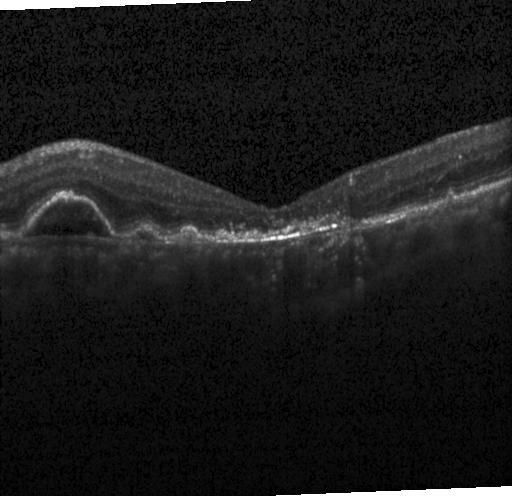
OCT B-scan. Diagnosis: a choroidal neovascular membrane.